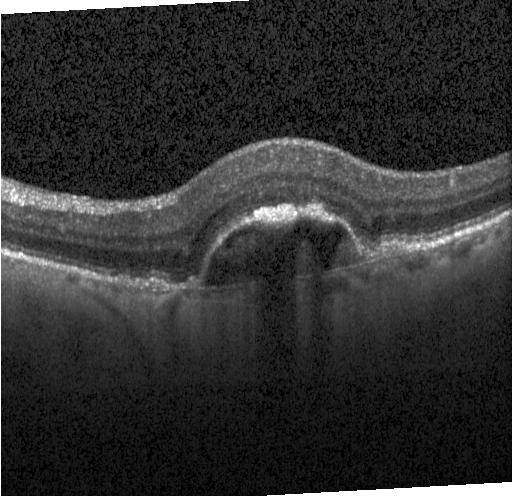 Dx: a choroidal neovascular membrane.